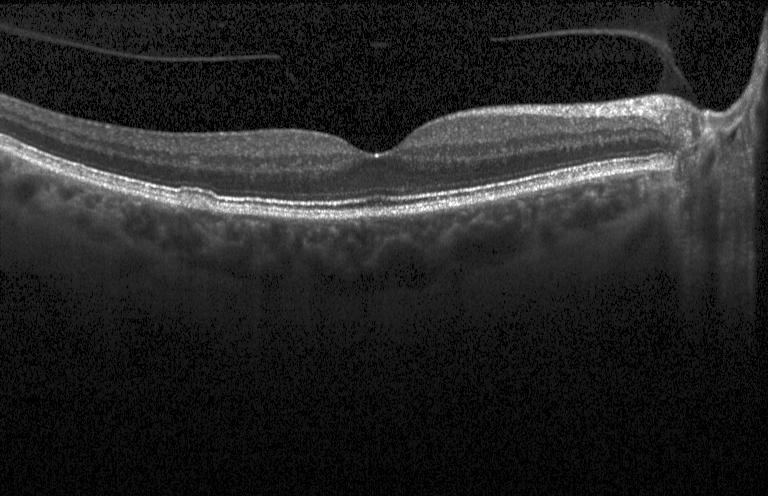 Through the macula. SD-OCT. Optical coherence tomography scan. Heidelberg Spectralis — Macular OCT: no evidence of choroidal neovascularization, diabetic macular edema, or drusen.